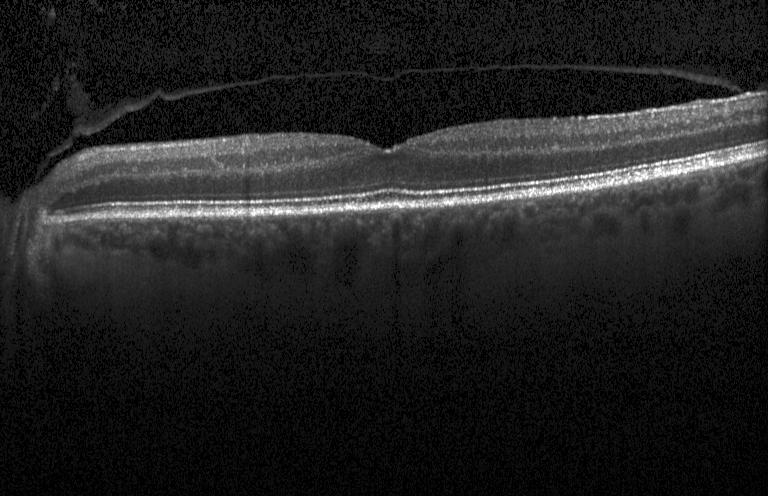

Spectral-domain optical coherence tomography, centered on the fovea, retinal OCT cross-section, acquired on a Heidelberg Spectralis.
Assessment: no choroidal neovascularization, diabetic macular edema, or drusen.